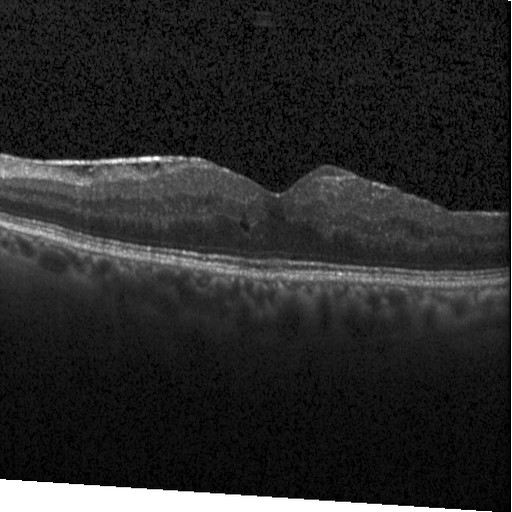

Optical coherence tomography B-scan. Spectral-domain OCT
The scan shows diabetic macular edema.